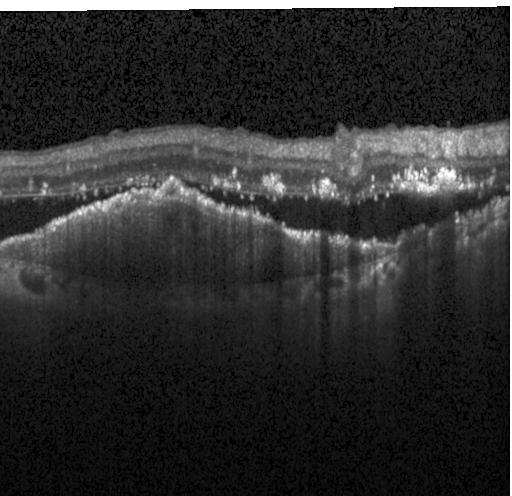 Centered on the fovea · spectral-domain OCT · retinal OCT B-scan · Heidelberg Spectralis OCT system — This B-scan demonstrates choroidal neovascularization (CNV).